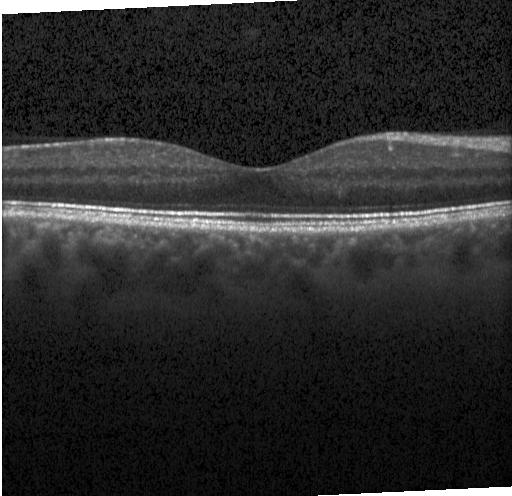 Retinal OCT B-scan. The scan shows neither choroidal neovascularization, diabetic macular edema, nor drusen.